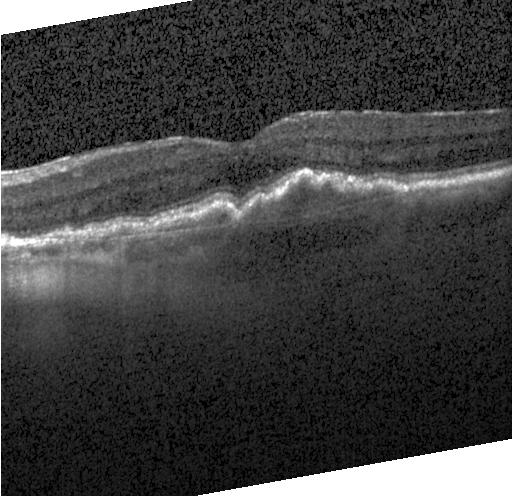

Assessment: choroidal neovascularization.